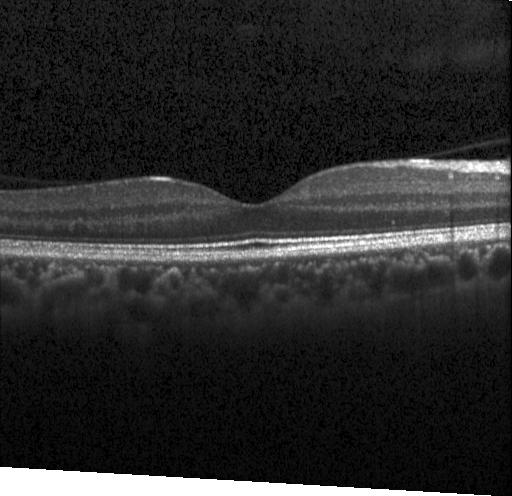
OCT B-scan, fovea-centered. Dx: no choroidal neovascularization, no diabetic macular edema, and no drusen.